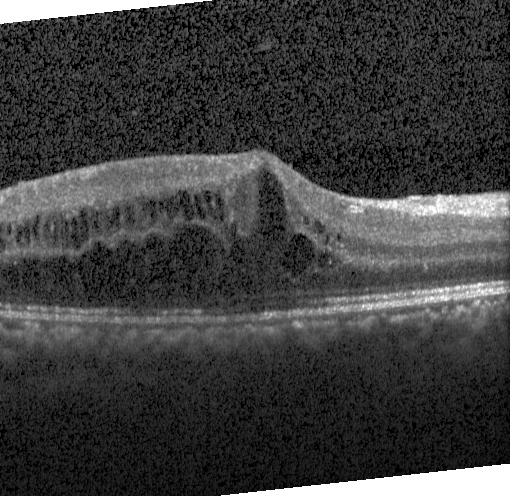

OCT finding: DME.